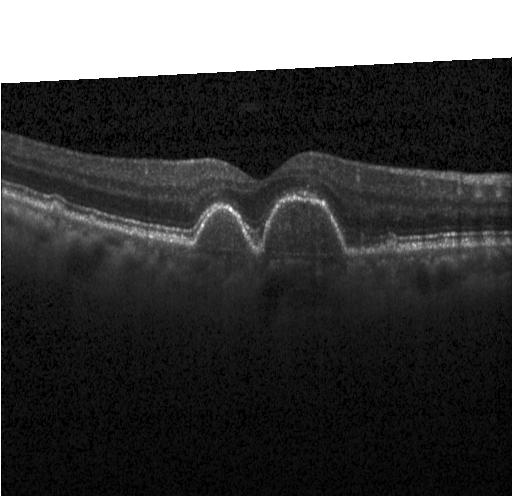 Instrument: Heidelberg Spectralis · OCT line scan.
Impression: drusen.